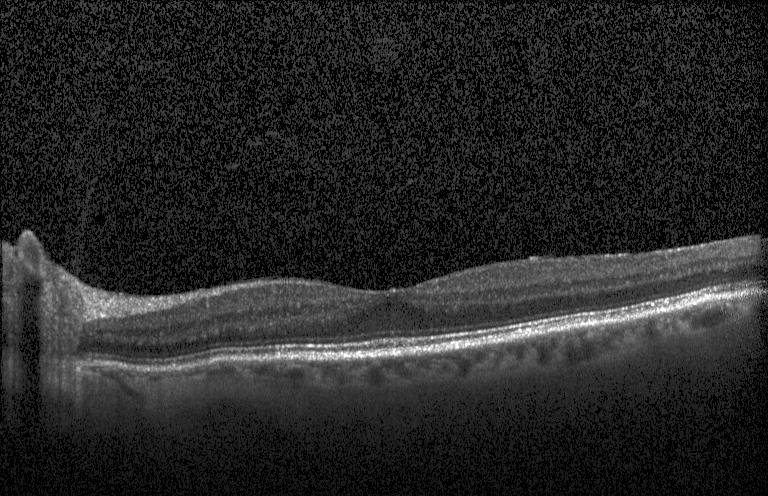

This B-scan demonstrates neither choroidal neovascularization, diabetic macular edema, nor drusen.